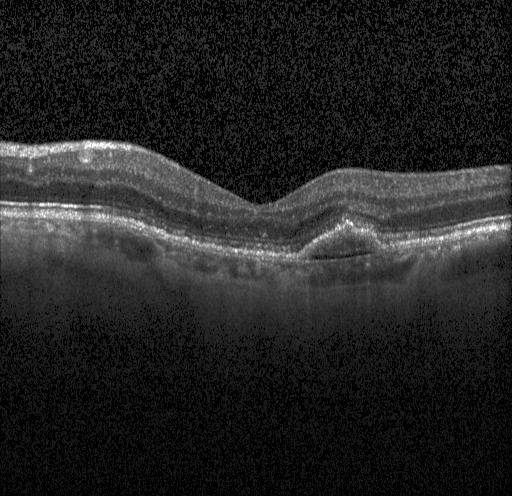

Centered on the fovea; OCT B-scan — Finding: CNV.